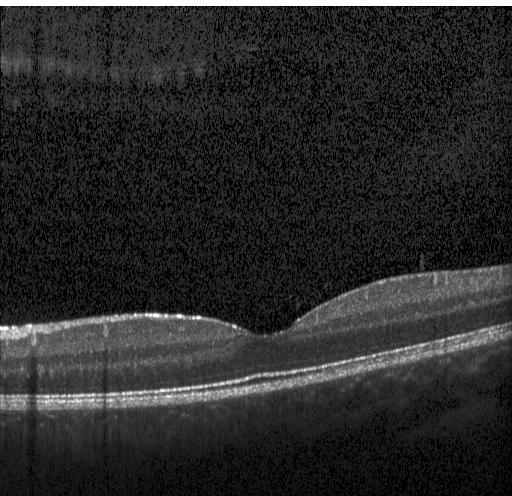 Through the macula, Heidelberg Spectralis, optical coherence tomography B-scan — Assessment: no choroidal neovascularization, no diabetic macular edema, and no drusen.